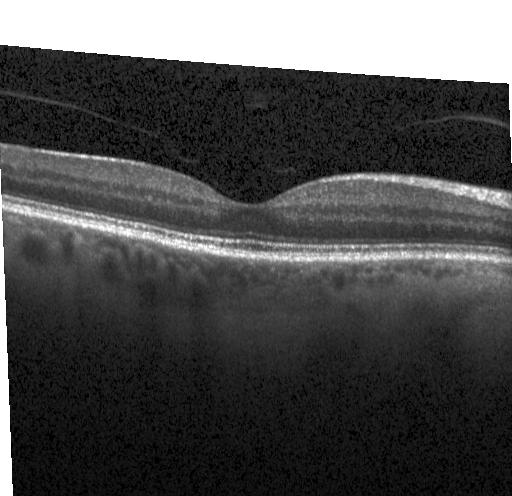
Retinal OCT B-scan; macular scan; instrument: Heidelberg Spectralis — This B-scan demonstrates neither choroidal neovascularization, diabetic macular edema, nor drusen.